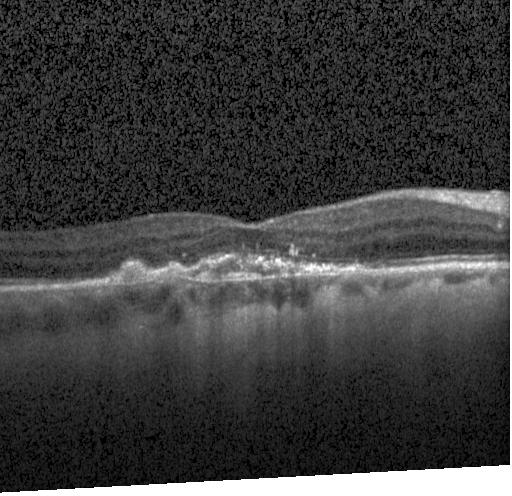 Diagnosis: choroidal neovascularization.